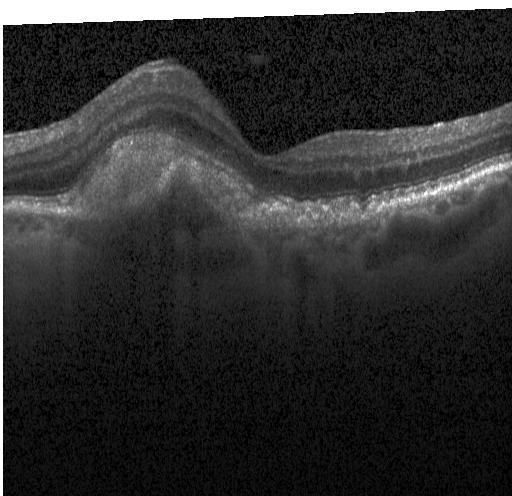 Finding: choroidal neovascularization.